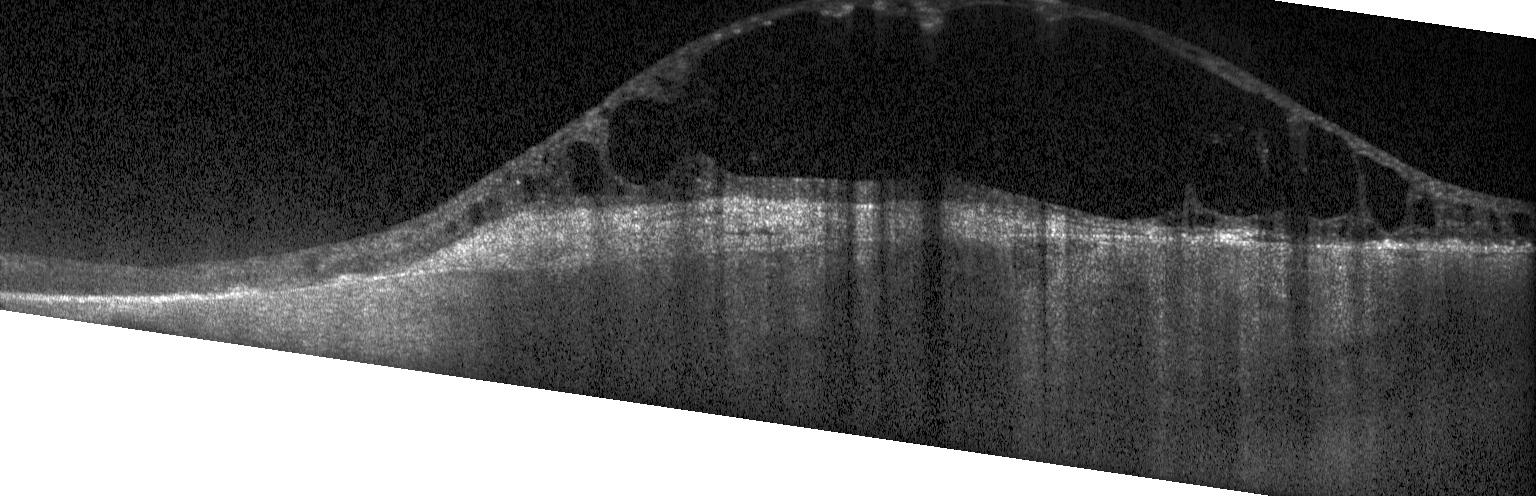

Spectral-domain OCT · retinal OCT cross-section · fovea-centered.
Macular OCT: choroidal neovascularization.